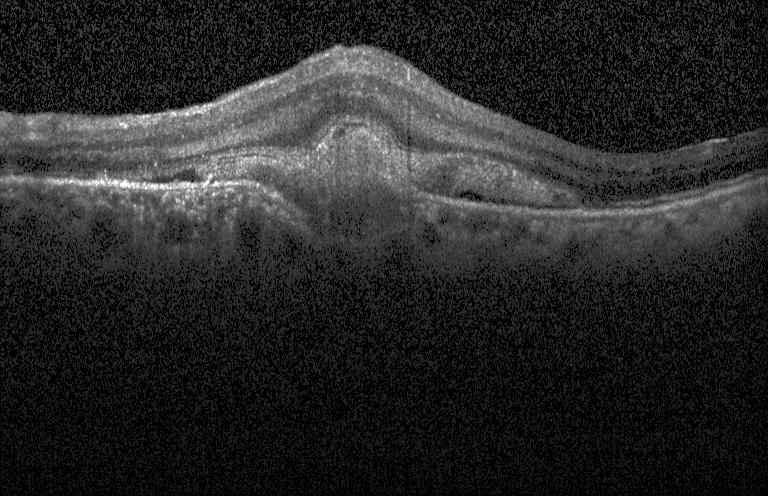
Diagnosis: a choroidal neovascular membrane.